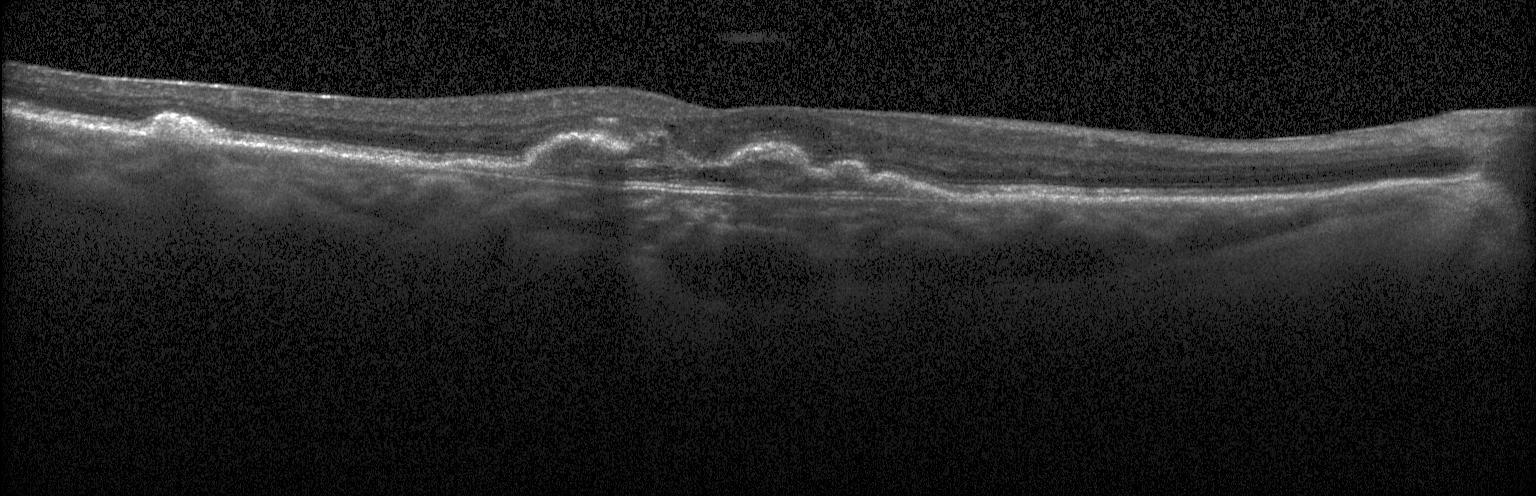 OCT B-scan, centered on the fovea, acquired on a Heidelberg Spectralis. Macular OCT: choroidal neovascularization (CNV).